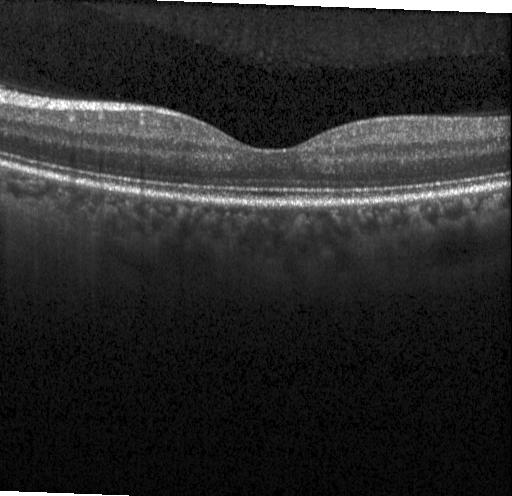 Fovea-centered; optical coherence tomography scan.
Assessment: no choroidal neovascularization, no diabetic macular edema, and no drusen.